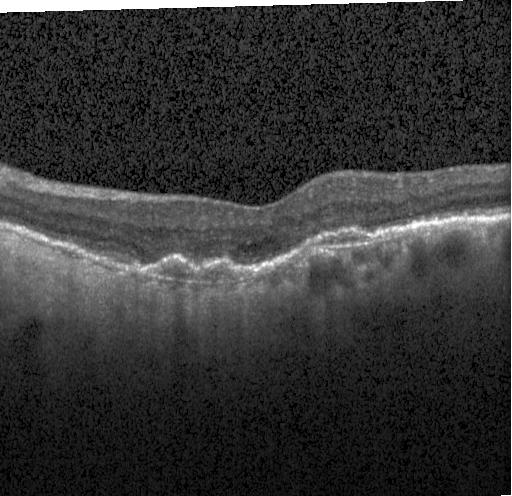 Heidelberg Spectralis; centered on the fovea; optical coherence tomography scan; spectral-domain optical coherence tomography — OCT finding: CNV.